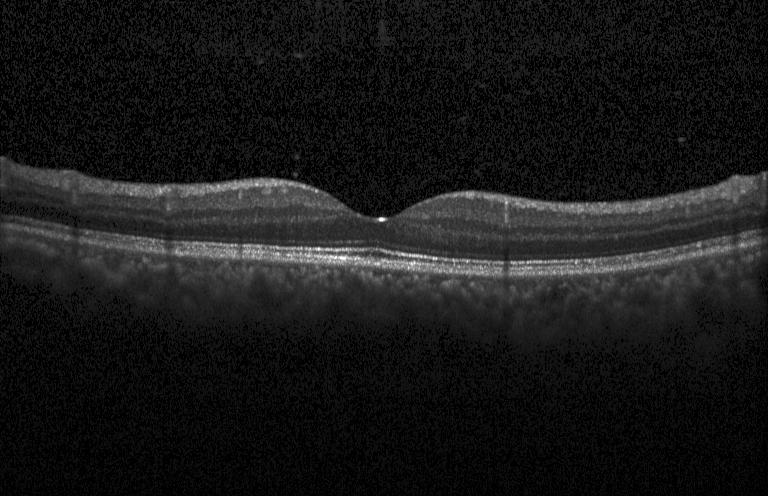
Horizontal scan through the fovea · SD-OCT · optical coherence tomography B-scan. OCT finding: neither choroidal neovascularization, diabetic macular edema, nor drusen.